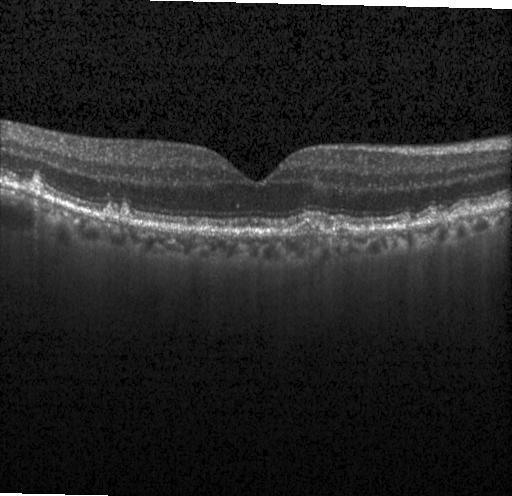 Optical coherence tomography B-scan
Multiple drusen.